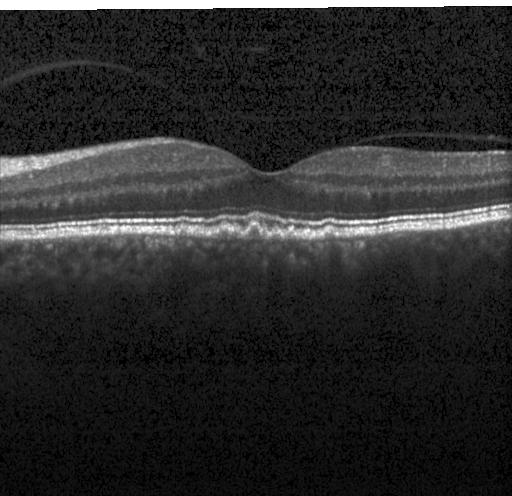
Macular OCT demonstrating sub-RPE drusenoid deposits.